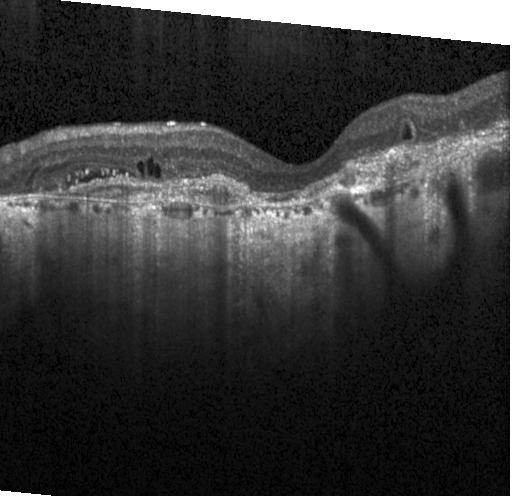

Macular OCT demonstrating a choroidal neovascular membrane.